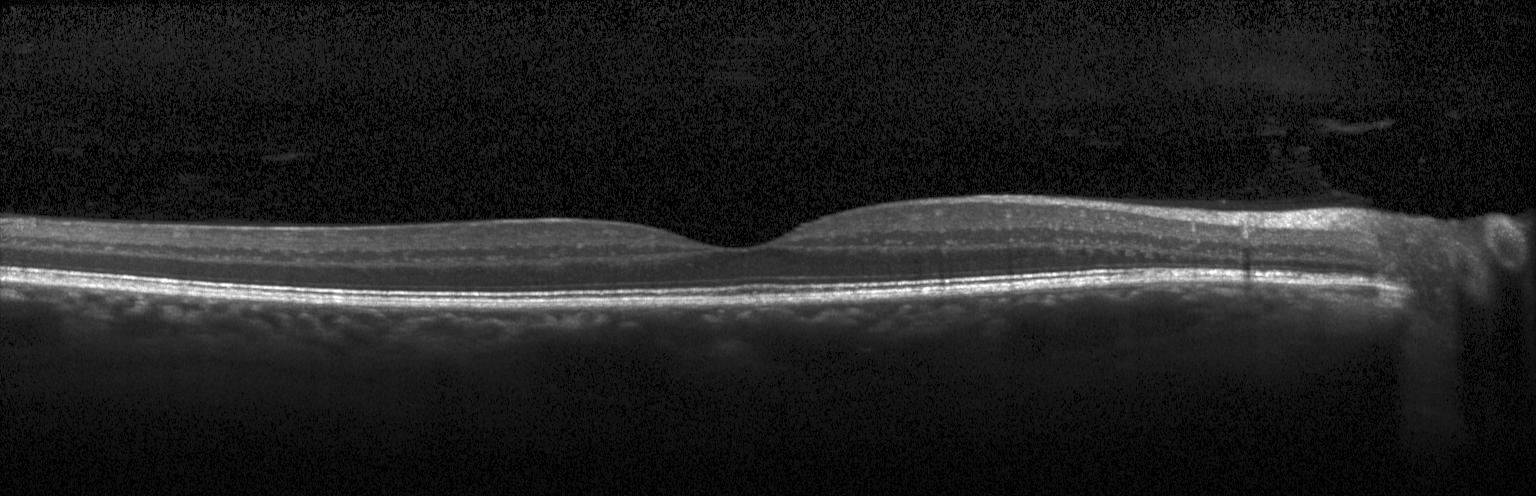 Diagnosis: no evidence of CNV, DME, or drusen.